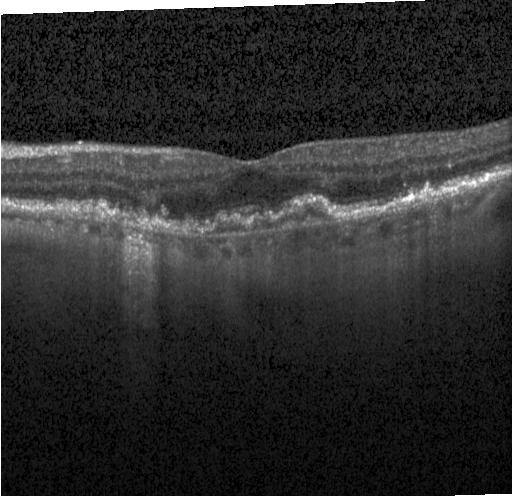 Centered on the fovea · spectral-domain optical coherence tomography · optical coherence tomography scan.
Finding: a choroidal neovascular membrane.